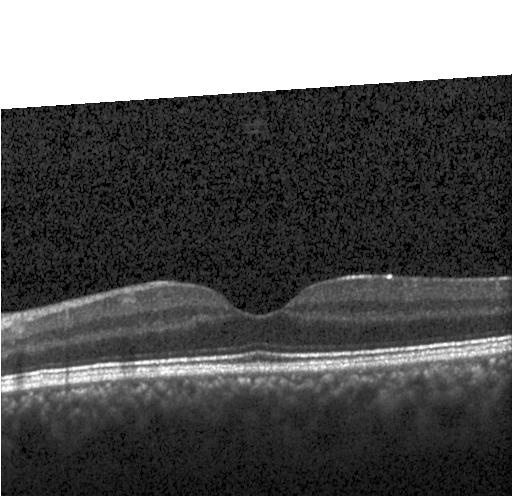
OCT B-scan — Finding: no evidence of choroidal neovascularization, diabetic macular edema, or drusen.